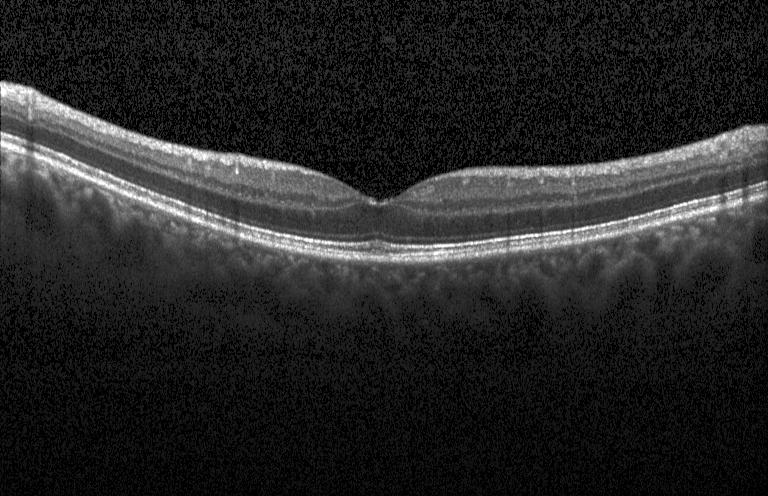

Macular OCT: neither choroidal neovascularization, diabetic macular edema, nor drusen.